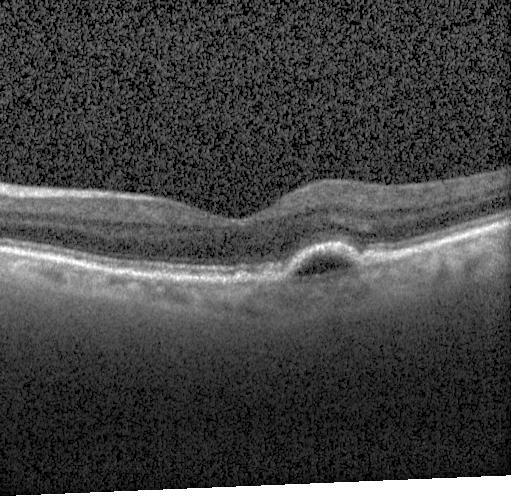

Spectral-domain optical coherence tomography; OCT line scan.
Assessment: a choroidal neovascular membrane.